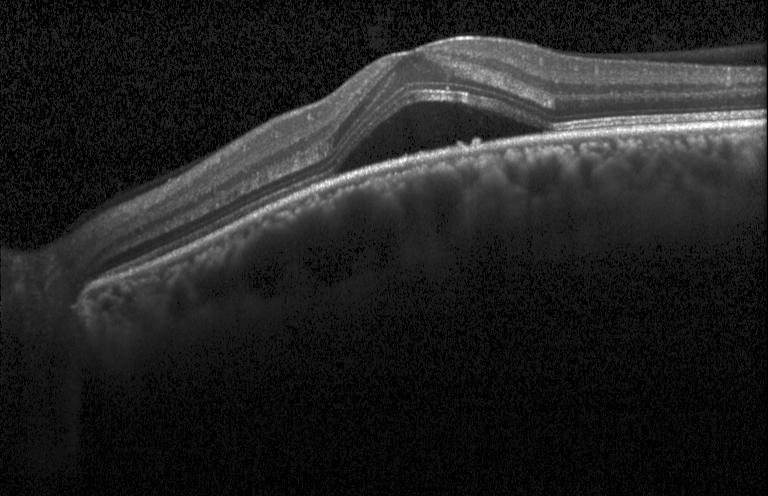
Finding: CNV.